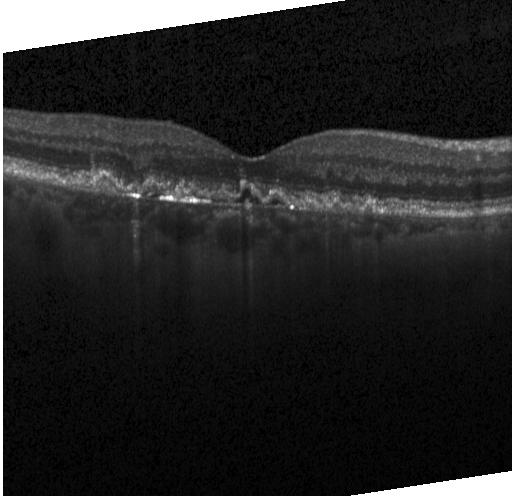
Spectral-domain optical coherence tomography · optical coherence tomography B-scan · macular scan — The scan shows CNV.